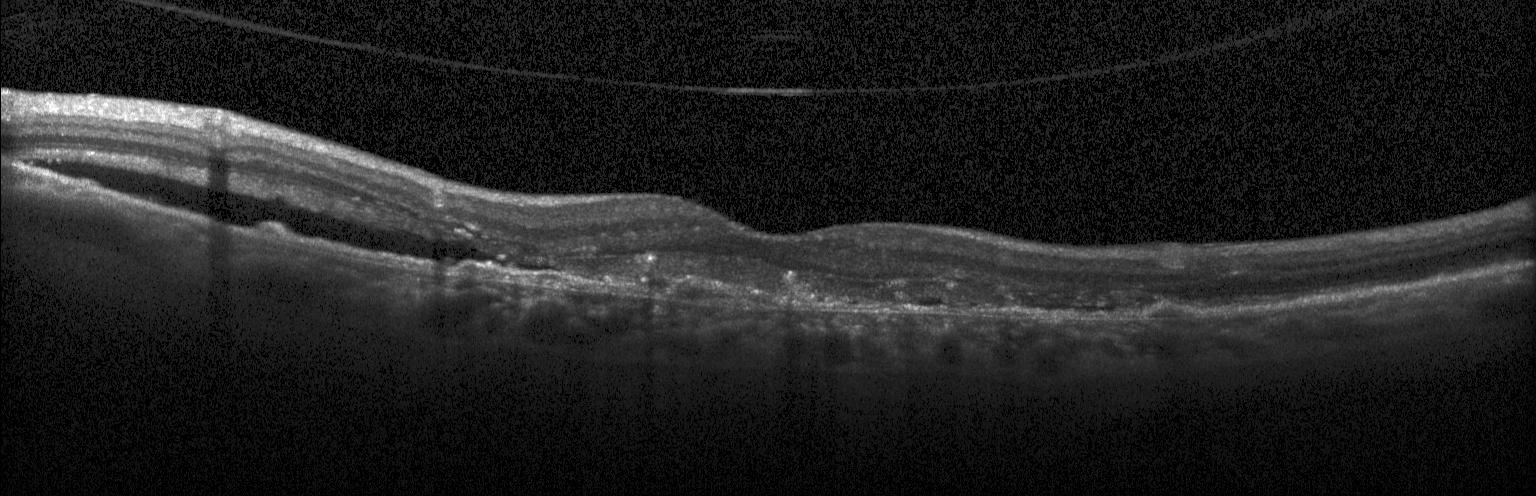
OCT B-scan showing CNV.